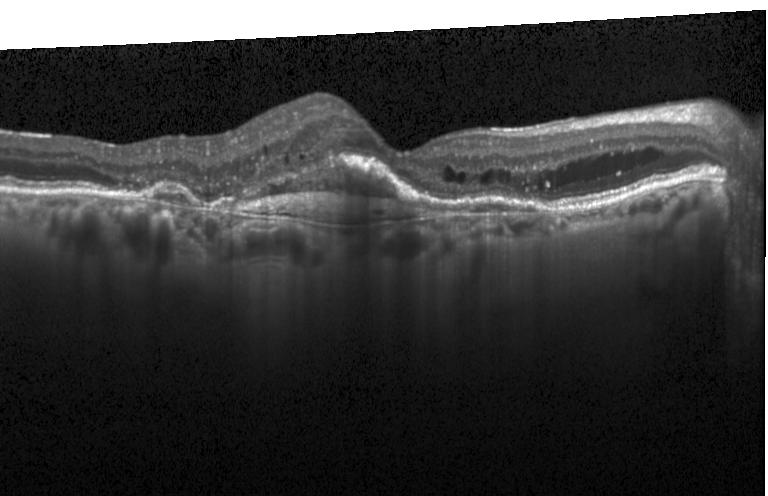 Retinal OCT cross-section, acquired on a Heidelberg Spectralis, SD-OCT — Diagnosis: a choroidal neovascular membrane.